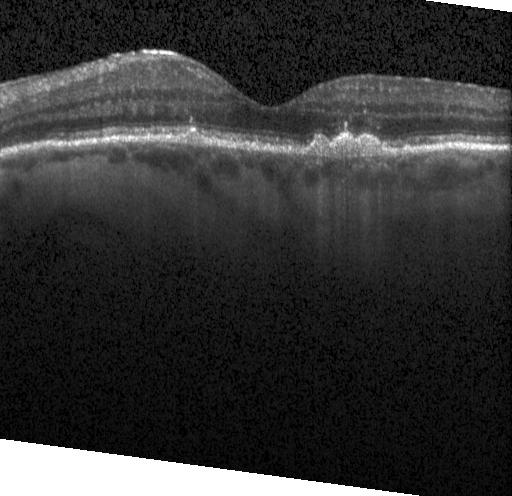

Macular OCT demonstrating sub-RPE drusenoid deposits.